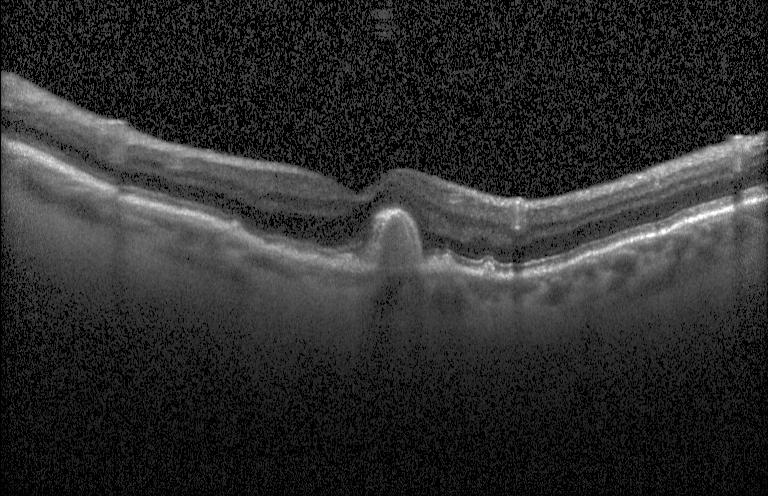 OCT B-scan showing sub-RPE drusenoid deposits.